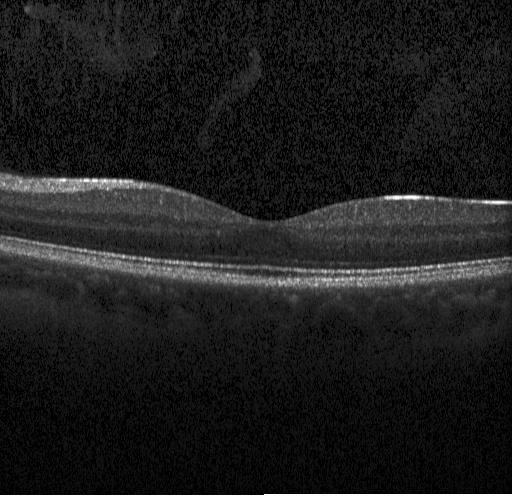 No choroidal neovascularization, diabetic macular edema, or drusen.